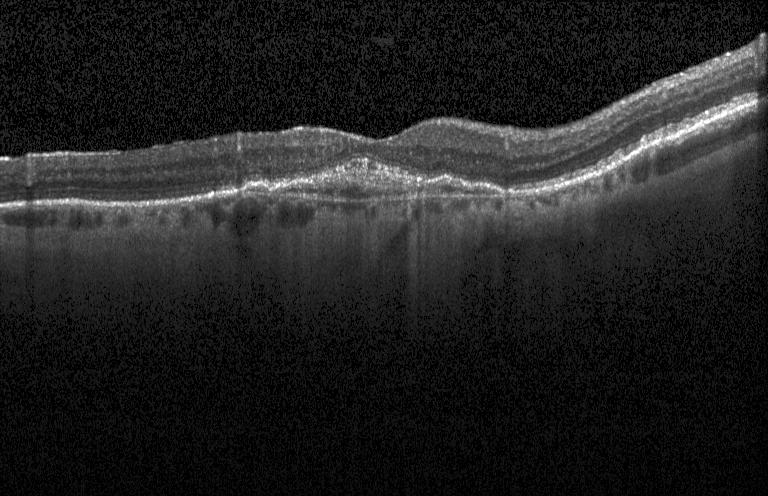

OCT finding: a choroidal neovascular membrane.